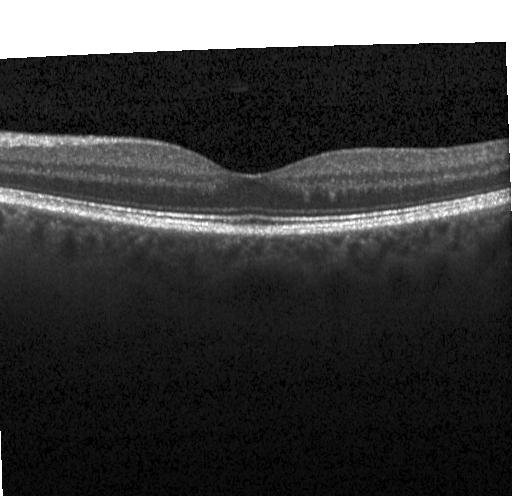 Centered on the fovea · retinal OCT B-scan · instrument: Heidelberg Spectralis — OCT finding: neither choroidal neovascularization, diabetic macular edema, nor drusen.